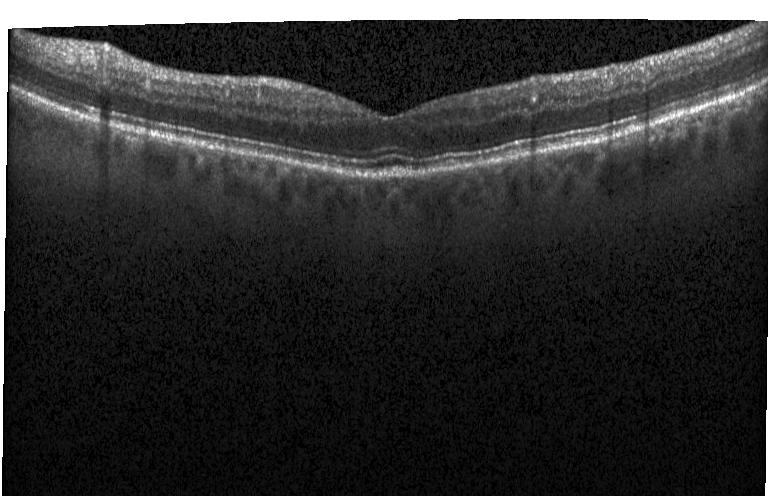
Dx: neither CNV, DME, nor drusen.